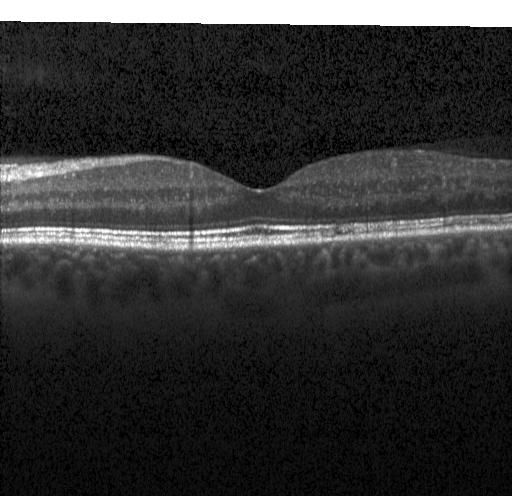

Retinal OCT cross-section
OCT finding: neither CNV, DME, nor drusen.